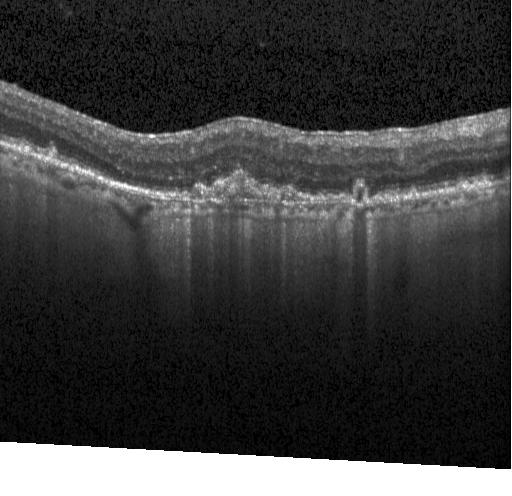 Finding: choroidal neovascularization (CNV).